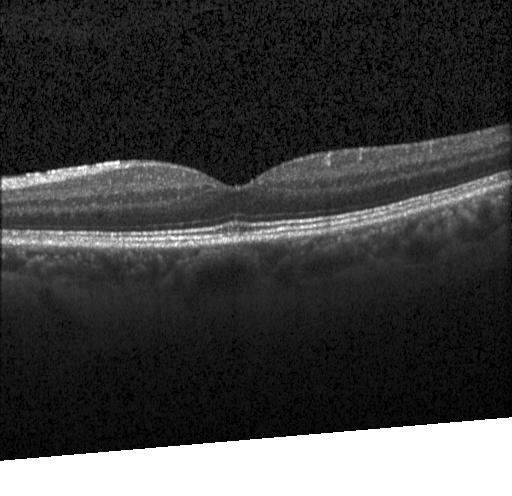

OCT B-scan; spectral-domain OCT; through the macula.
Assessment: no evidence of choroidal neovascularization, diabetic macular edema, or drusen.